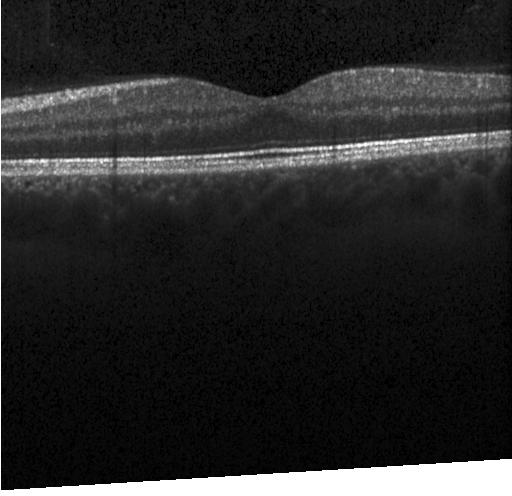
Assessment: neither choroidal neovascularization, diabetic macular edema, nor drusen.